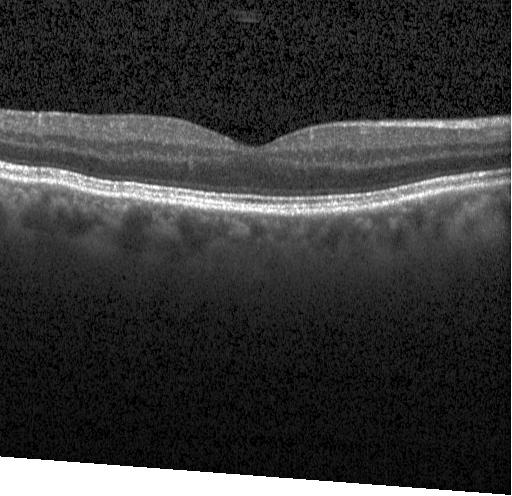
Retinal OCT cross-section; Heidelberg Spectralis OCT system; SD-OCT; horizontal scan through the fovea
Impression: no CNV, DME, or drusen.